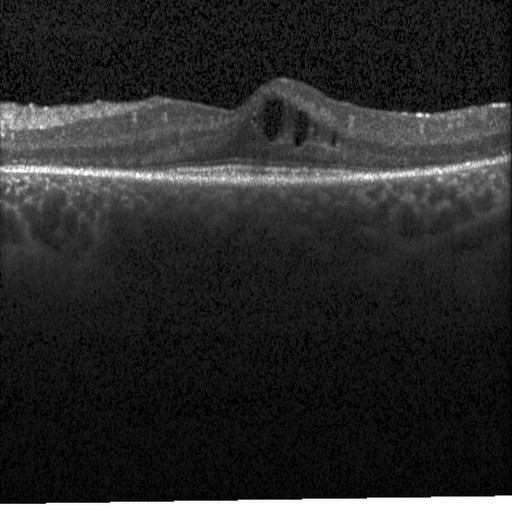 Retinal OCT B-scan. Spectral-domain OCT. Dx: diabetic macular edema (DME).